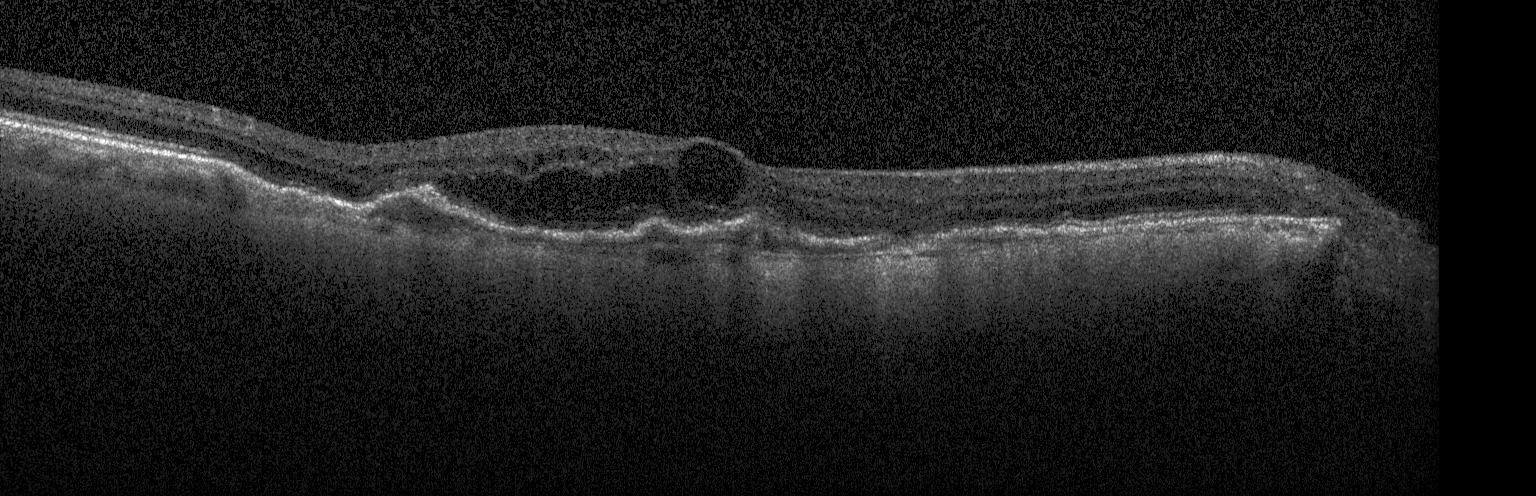 Spectral-domain OCT. Through the macula. Optical coherence tomography scan — Diagnosis: choroidal neovascularization.